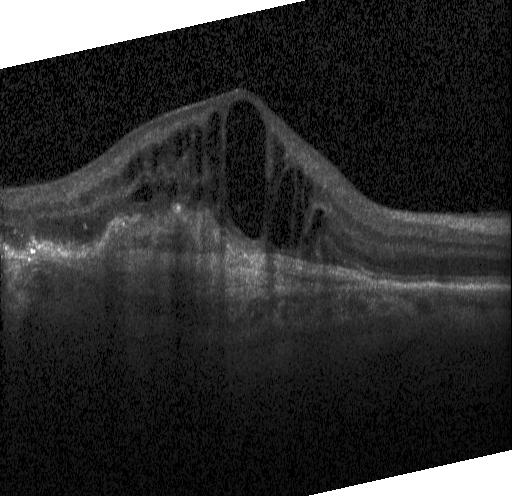

Instrument: Heidelberg Spectralis; optical coherence tomography B-scan; horizontal scan through the fovea; SD-OCT
This B-scan demonstrates choroidal neovascularization (CNV).